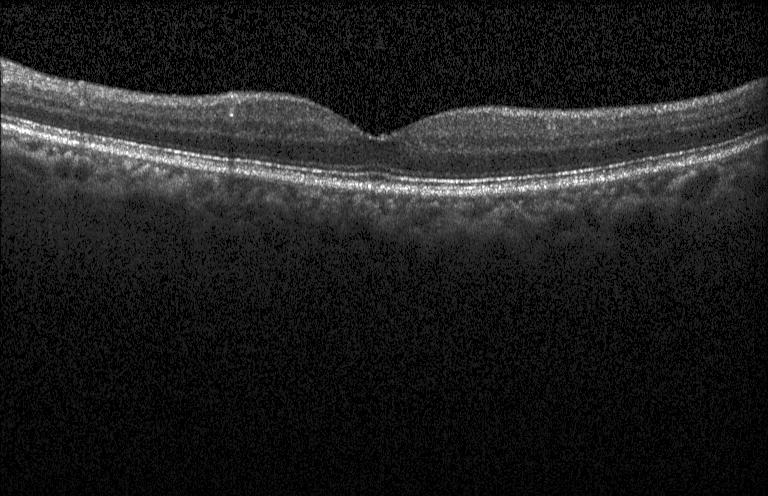
OCT B-scan; horizontal scan through the fovea.
No choroidal neovascularization, no diabetic macular edema, and no drusen.